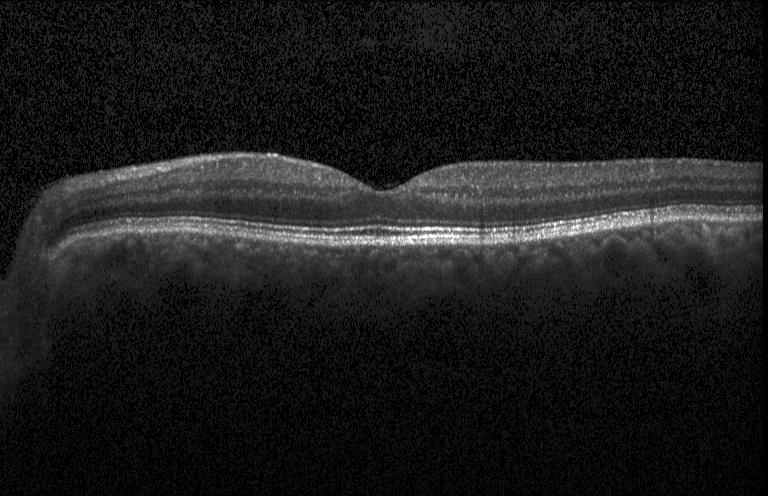

Retinal OCT B-scan. The scan shows no evidence of choroidal neovascularization, diabetic macular edema, or drusen.